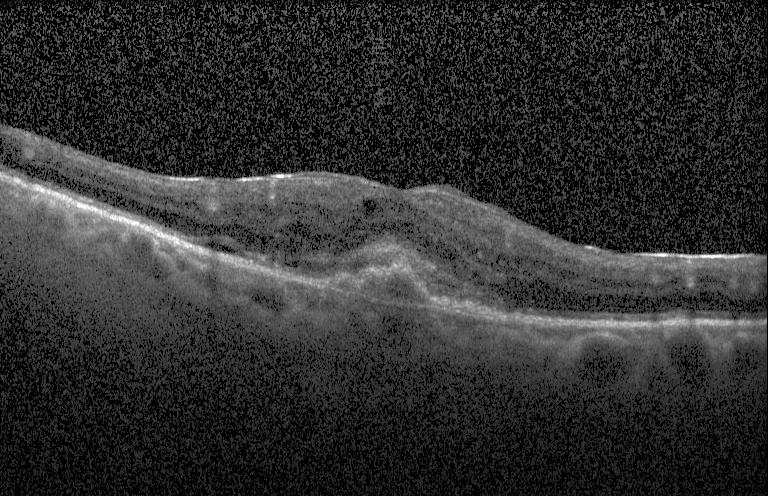 OCT B-scan. Spectral-domain optical coherence tomography. Heidelberg Spectralis. Impression: a choroidal neovascular membrane.